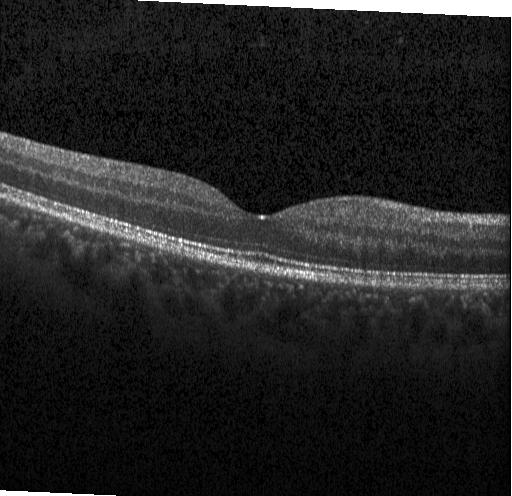
Macular OCT demonstrating neither CNV, DME, nor drusen.